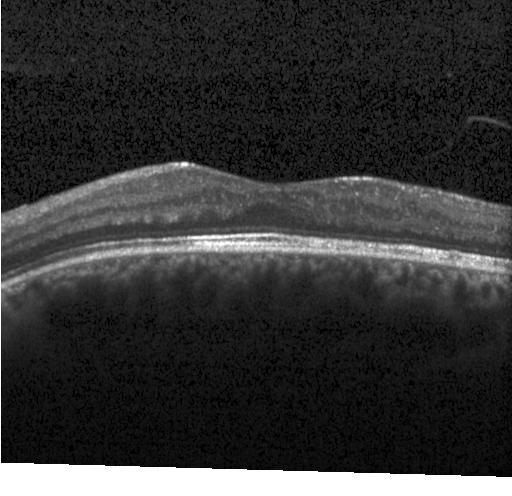 Retinal OCT B-scan.
OCT finding: no CNV, DME, or drusen.